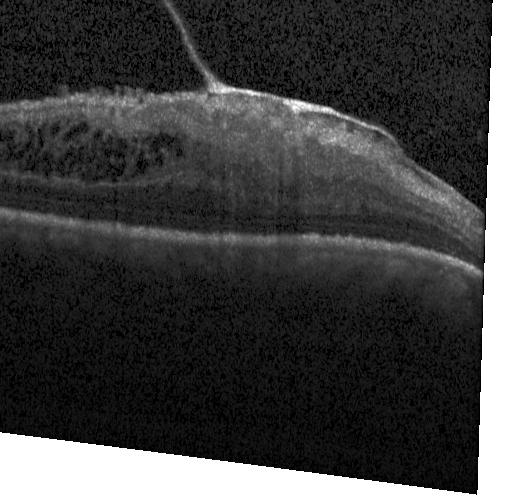 Retinal OCT B-scan — Dx: DME.